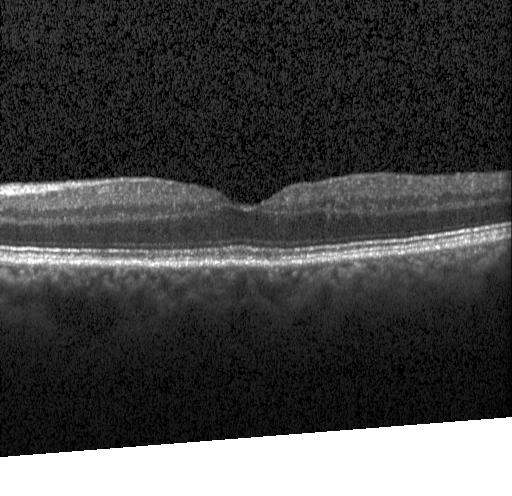 Spectral-domain optical coherence tomography. OCT B-scan. Heidelberg Spectralis OCT system. Diagnosis: neither choroidal neovascularization, diabetic macular edema, nor drusen.